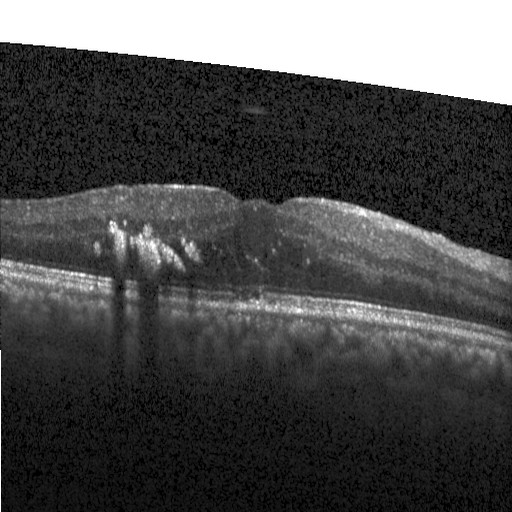 Impression: diabetic macular edema.